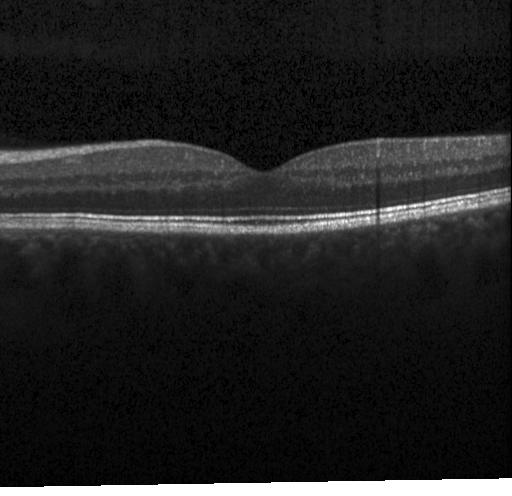

The scan shows no evidence of choroidal neovascularization, diabetic macular edema, or drusen.